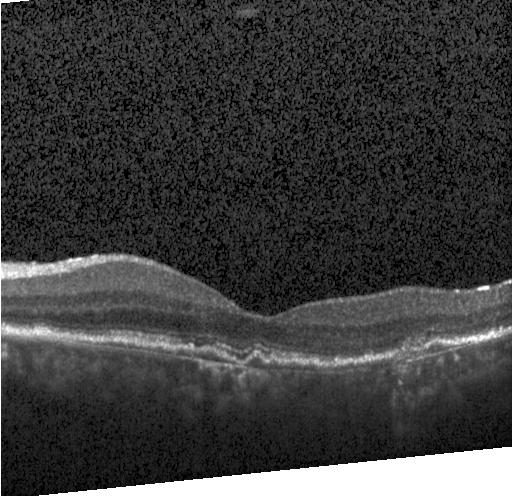
OCT finding: choroidal neovascularization (CNV).